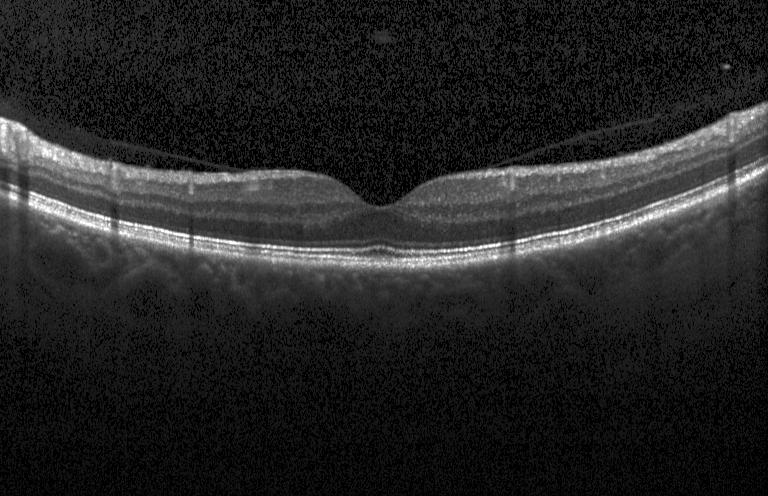 Heidelberg Spectralis · OCT B-scan
The scan shows no CNV, no DME, and no drusen.